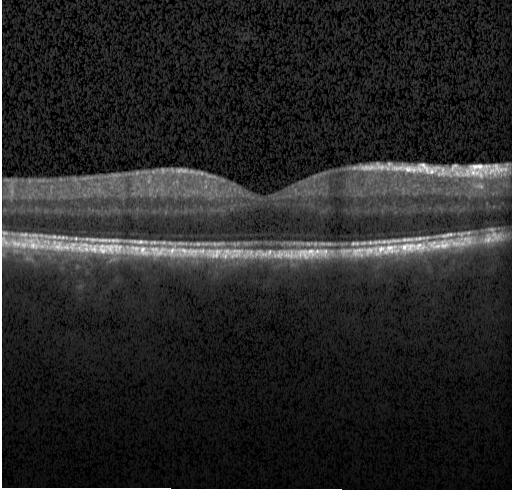 Heidelberg Spectralis OCT system · optical coherence tomography scan · spectral-domain optical coherence tomography · horizontal scan through the fovea. Macular OCT: no choroidal neovascularization, diabetic macular edema, or drusen.